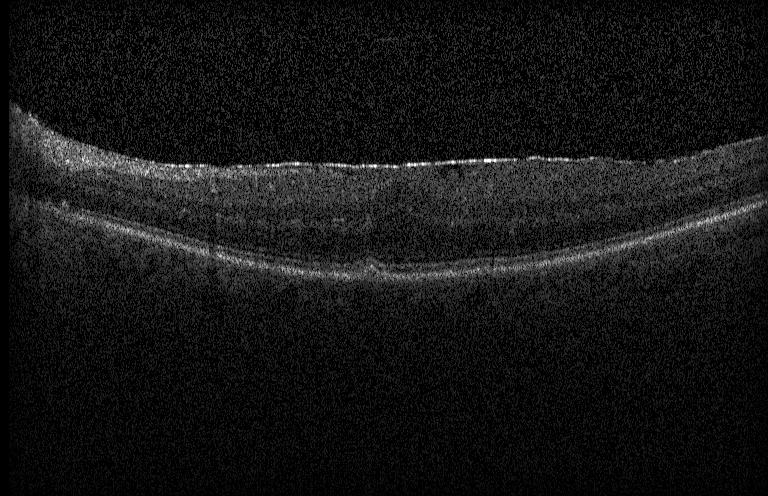
OCT B-scan; spectral-domain OCT; Heidelberg Spectralis; centered on the fovea — This B-scan demonstrates drusen.